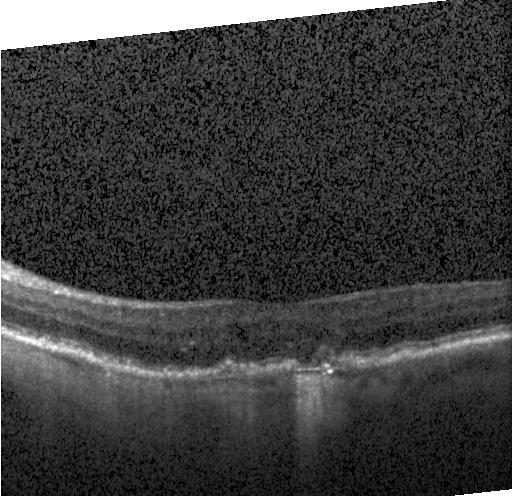
Heidelberg Spectralis · OCT B-scan — Impression: a choroidal neovascular membrane.